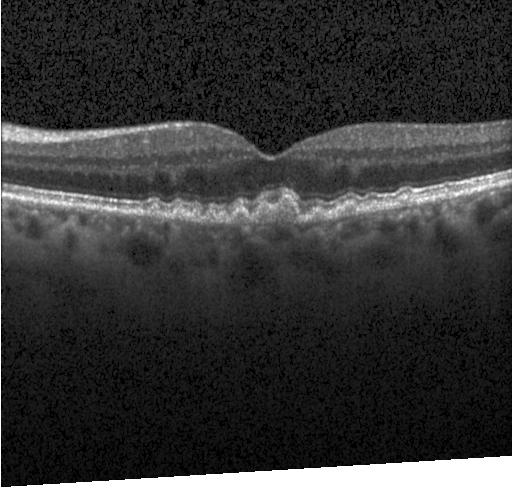 Retinal OCT cross-section · spectral-domain optical coherence tomography · macular scan · Heidelberg Spectralis.
OCT finding: drusen.